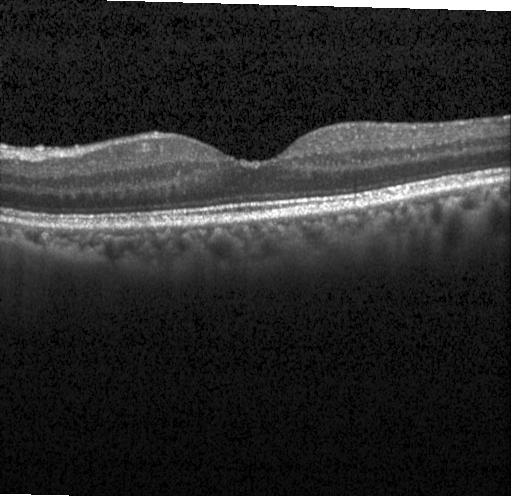 Diagnosis: neither choroidal neovascularization, diabetic macular edema, nor drusen.